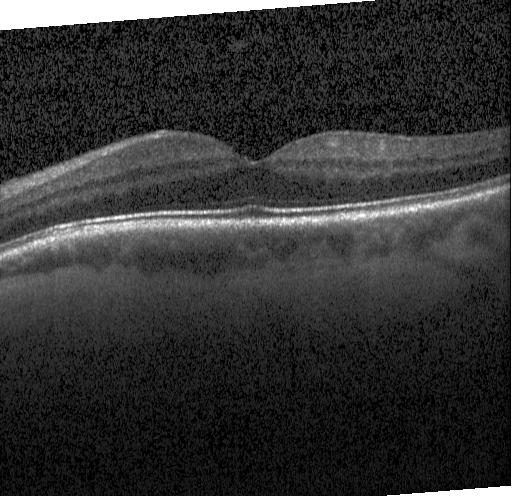 OCT line scan, through the macula, Heidelberg Spectralis, SD-OCT.
Macular OCT: neither choroidal neovascularization, diabetic macular edema, nor drusen.